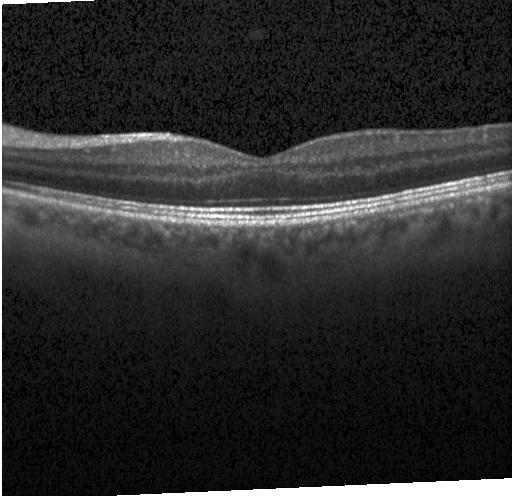

Retinal OCT cross-section, macular scan, SD-OCT, Heidelberg Spectralis OCT system — No choroidal neovascularization, diabetic macular edema, or drusen.